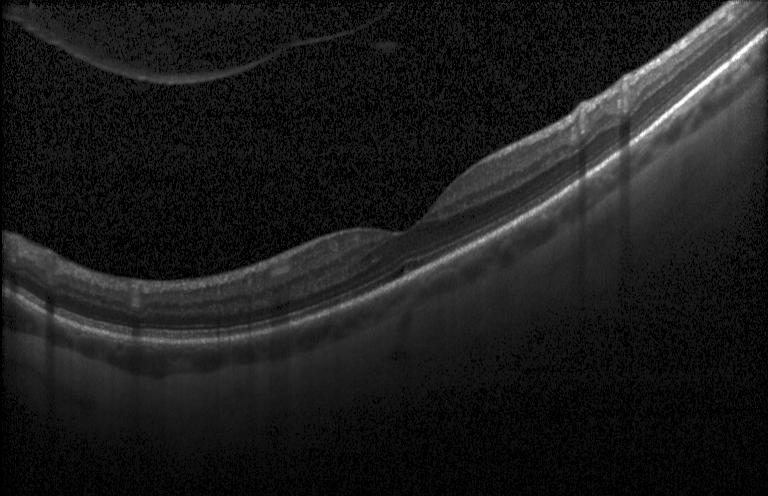
Fovea-centered. SD-OCT. Retinal OCT B-scan. Acquired on a Heidelberg Spectralis.
Neither CNV, DME, nor drusen.